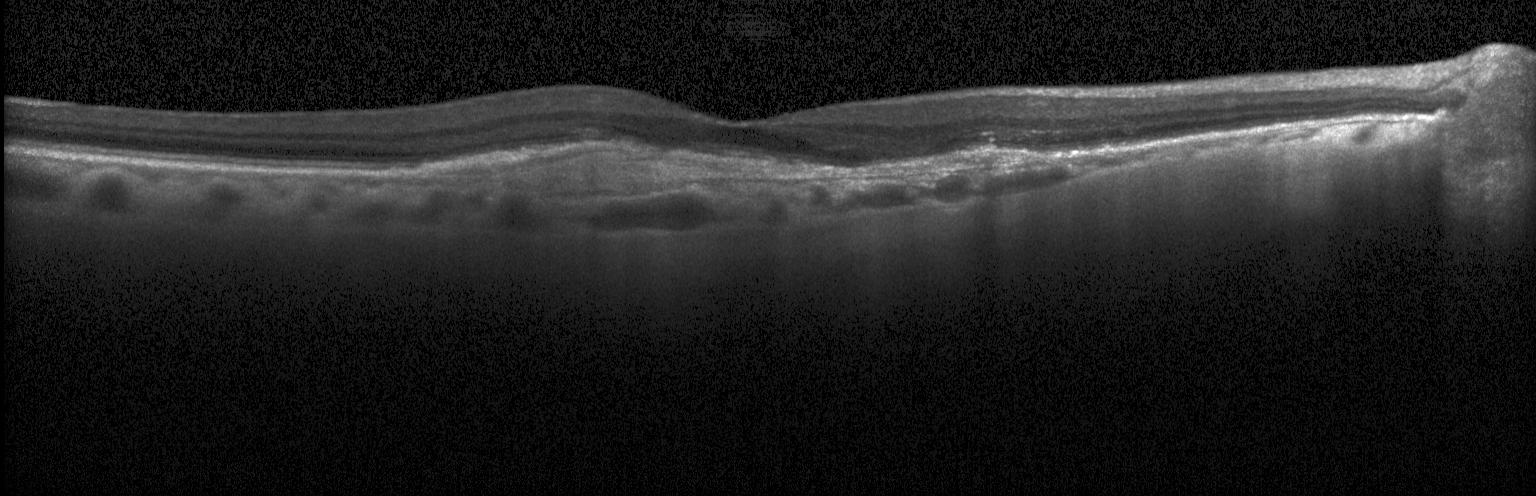 Diagnosis: a choroidal neovascular membrane.